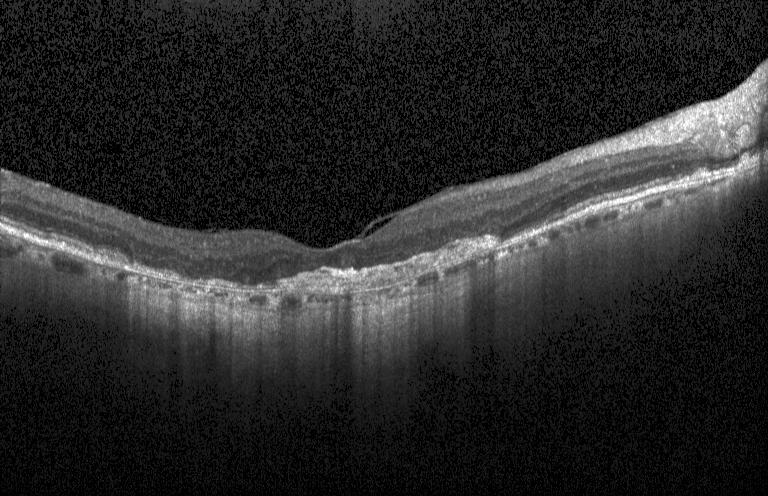 Impression: a choroidal neovascular membrane.